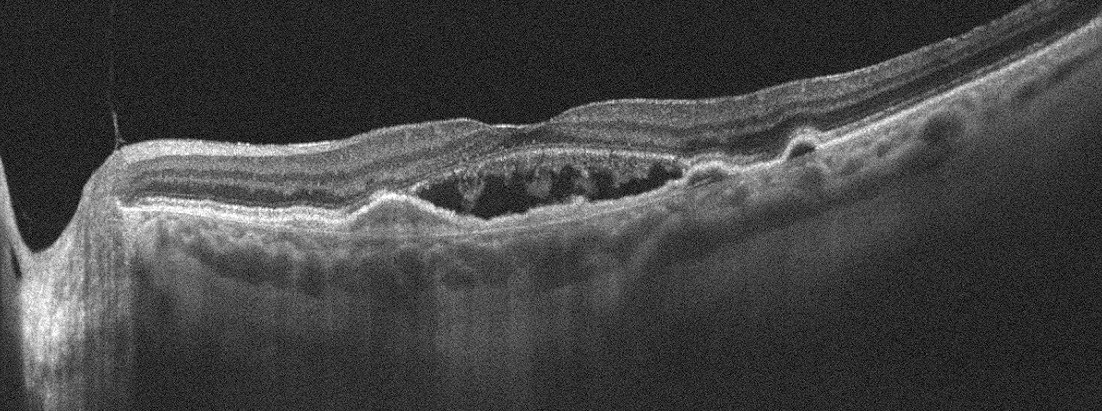 Retinal OCT B-scan — The scan shows age-related macular degeneration.